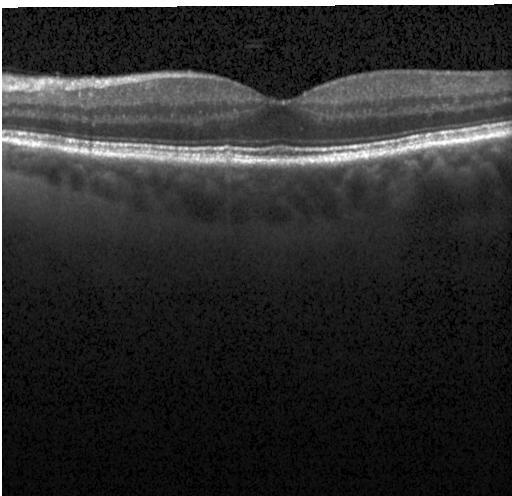
Neither choroidal neovascularization, diabetic macular edema, nor drusen.